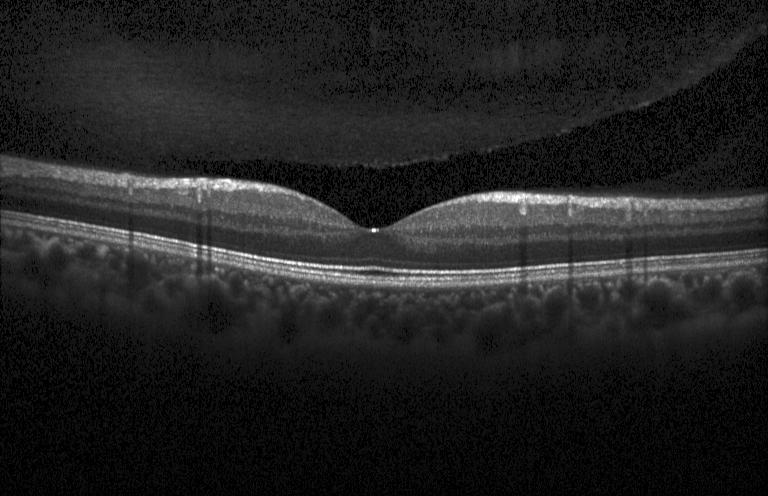

Retinal OCT cross-section
Dx: no evidence of choroidal neovascularization, diabetic macular edema, or drusen.